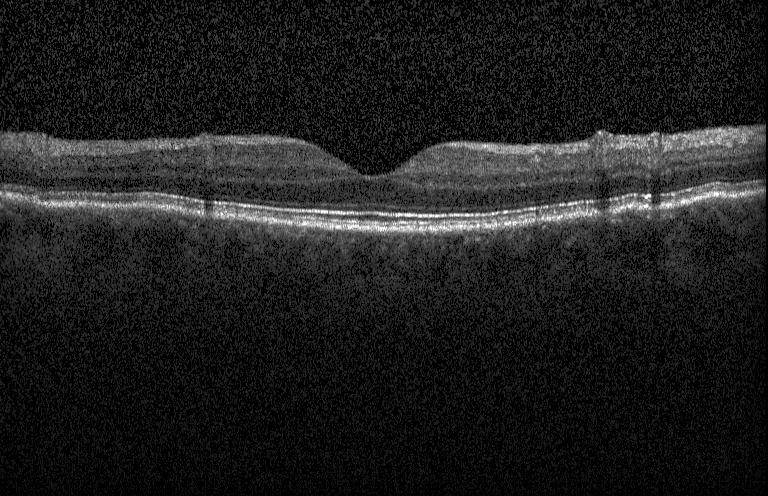

Diagnosis: no CNV, DME, or drusen.